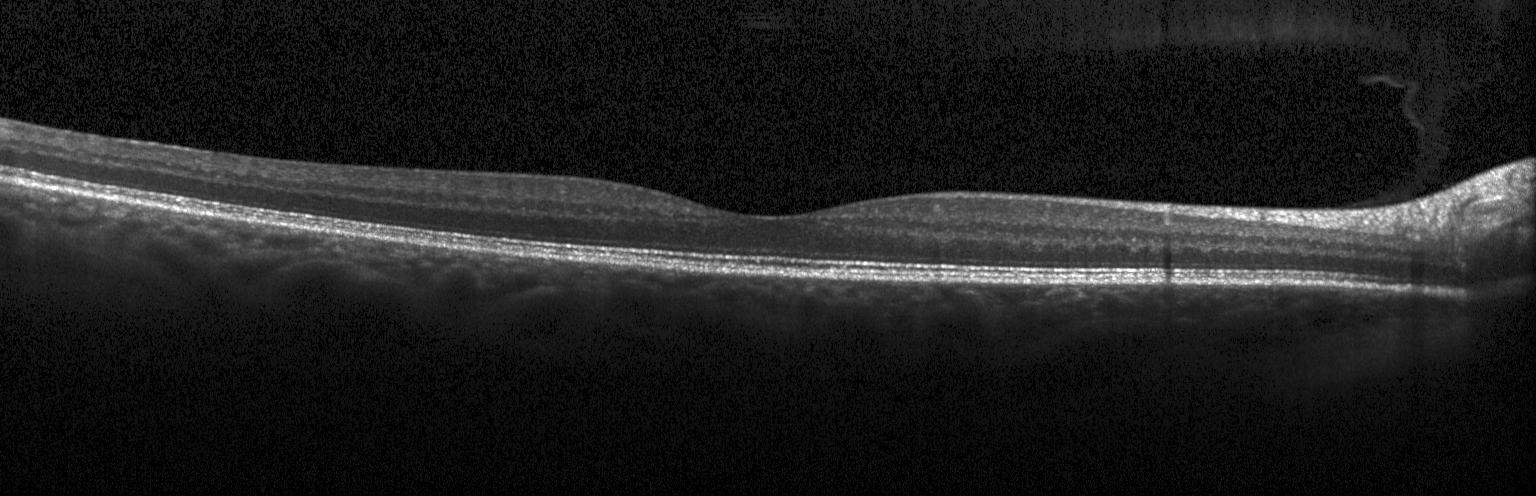

OCT B-scan — Finding: no CNV, DME, or drusen.